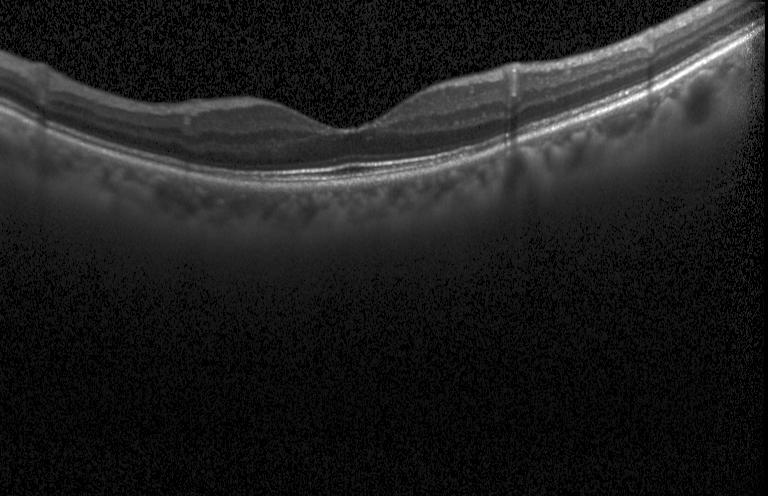

Diagnosis: no CNV, DME, or drusen.